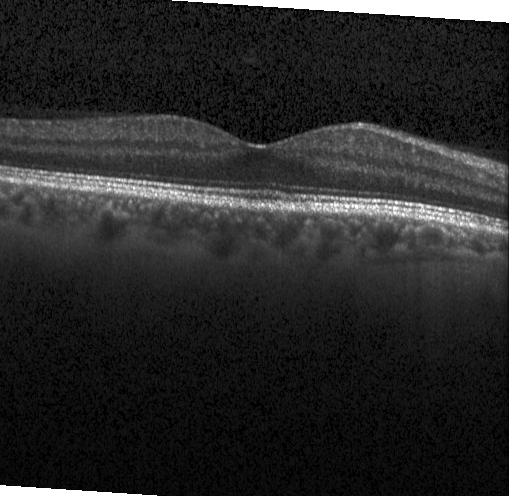 Spectral-domain OCT · optical coherence tomography B-scan — Finding: neither CNV, DME, nor drusen.